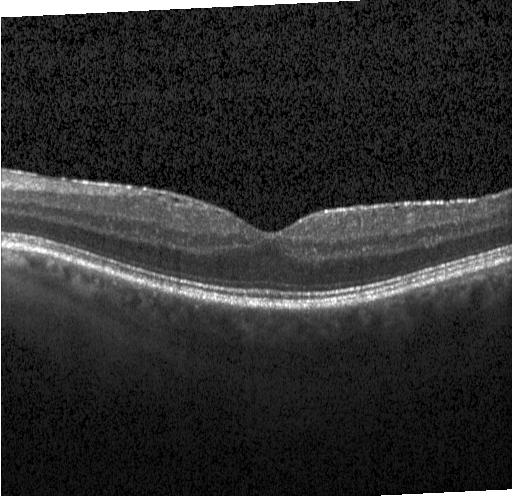

Heidelberg Spectralis; spectral-domain optical coherence tomography; through the macula; OCT line scan
Finding: no choroidal neovascularization, diabetic macular edema, or drusen.